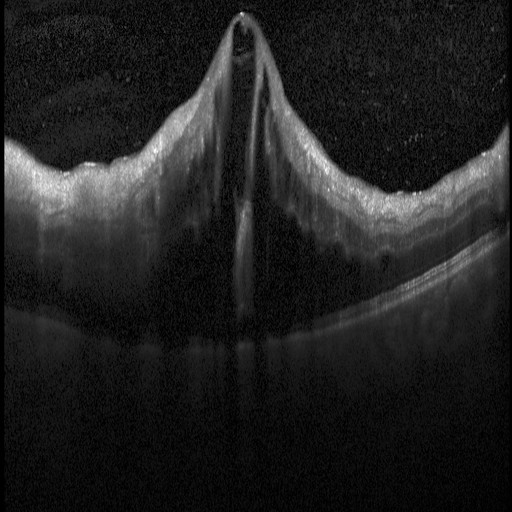 OCT line scan. Spectral-domain optical coherence tomography.
Diabetic macular edema.